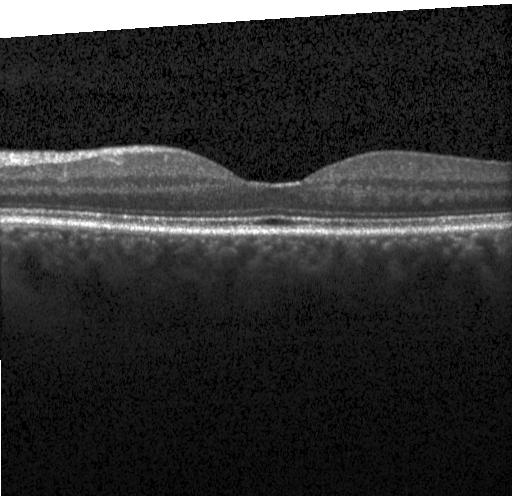
SD-OCT · OCT line scan · horizontal scan through the fovea · instrument: Heidelberg Spectralis. Finding: neither choroidal neovascularization, diabetic macular edema, nor drusen.